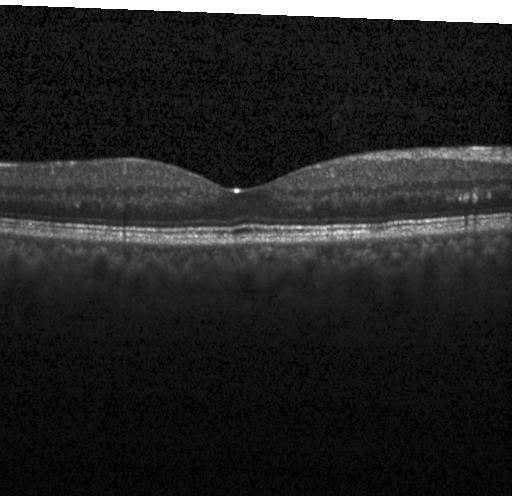 Spectral-domain OCT B-scan: neither CNV, DME, nor drusen.